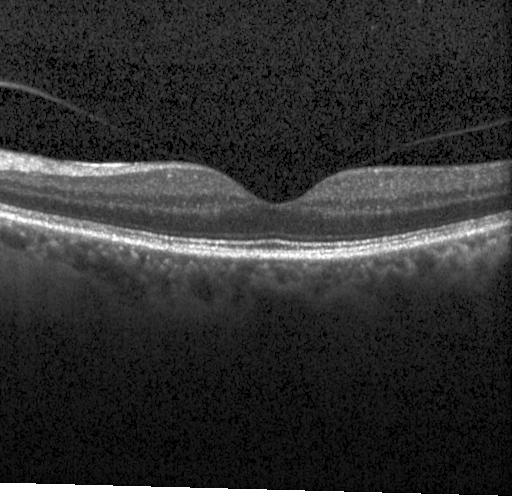
Instrument: Heidelberg Spectralis. Optical coherence tomography B-scan. Spectral-domain OCT. Horizontal scan through the fovea. Neither choroidal neovascularization, diabetic macular edema, nor drusen.